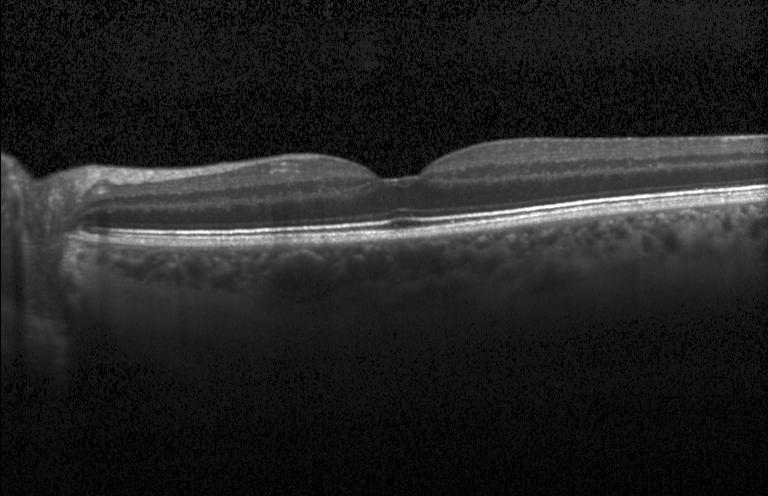 Retinal OCT B-scan; spectral-domain OCT; fovea-centered; acquired on a Heidelberg Spectralis
Impression: no choroidal neovascularization, diabetic macular edema, or drusen.